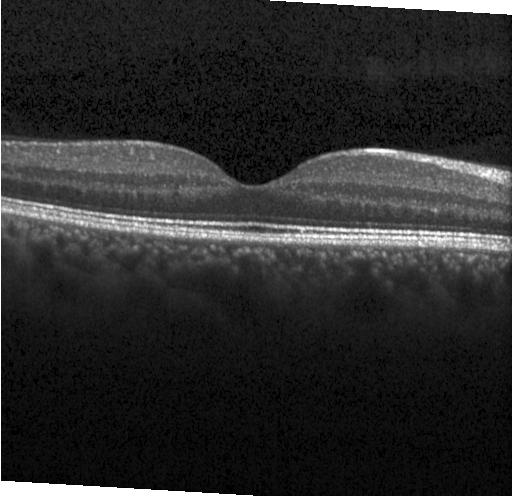 Finding: no choroidal neovascularization, diabetic macular edema, or drusen.